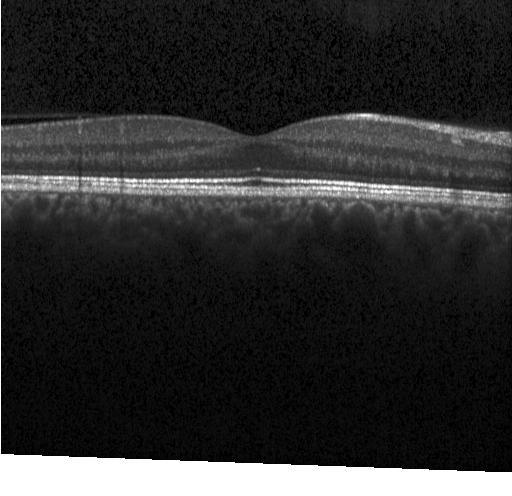

Finding: no evidence of CNV, DME, or drusen.